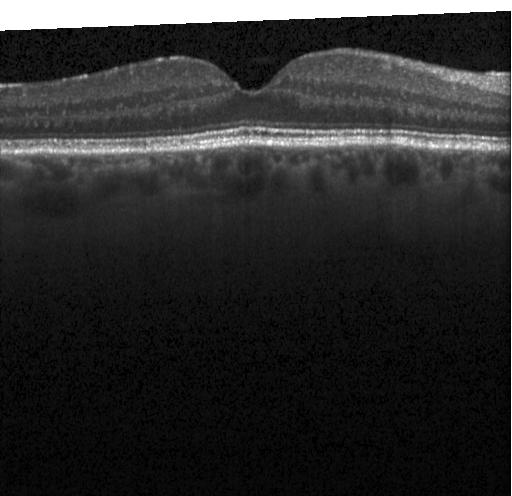 Retinal OCT cross-section
This B-scan demonstrates no choroidal neovascularization, diabetic macular edema, or drusen.